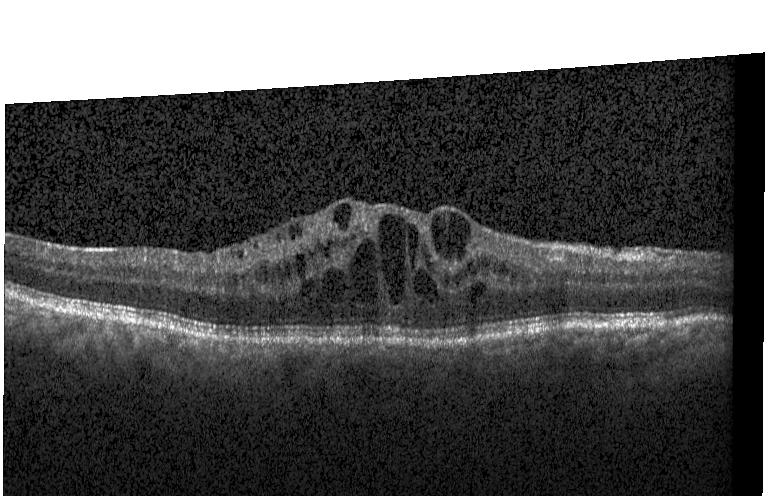
OCT B-scan, through the macula. Diagnosis: DME.